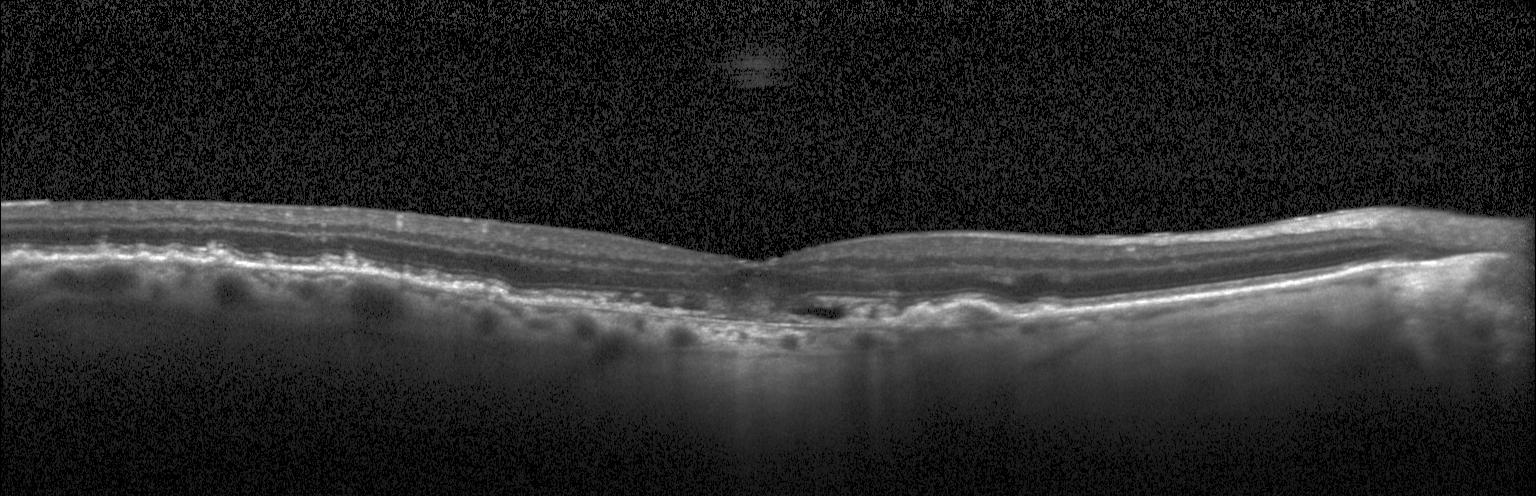 Heidelberg Spectralis OCT system · centered on the fovea · OCT line scan
Assessment: CNV.